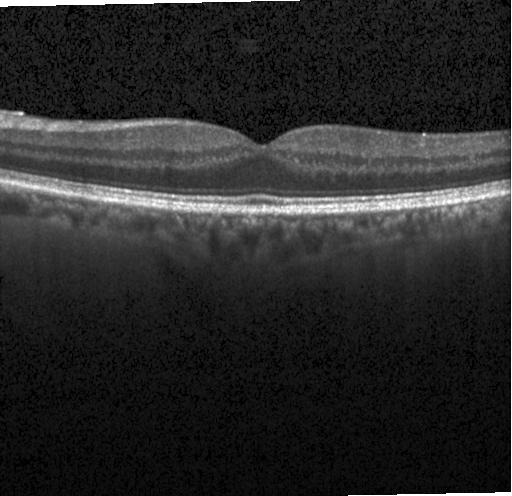

Macular scan, OCT B-scan
Impression: no CNV, no DME, and no drusen.